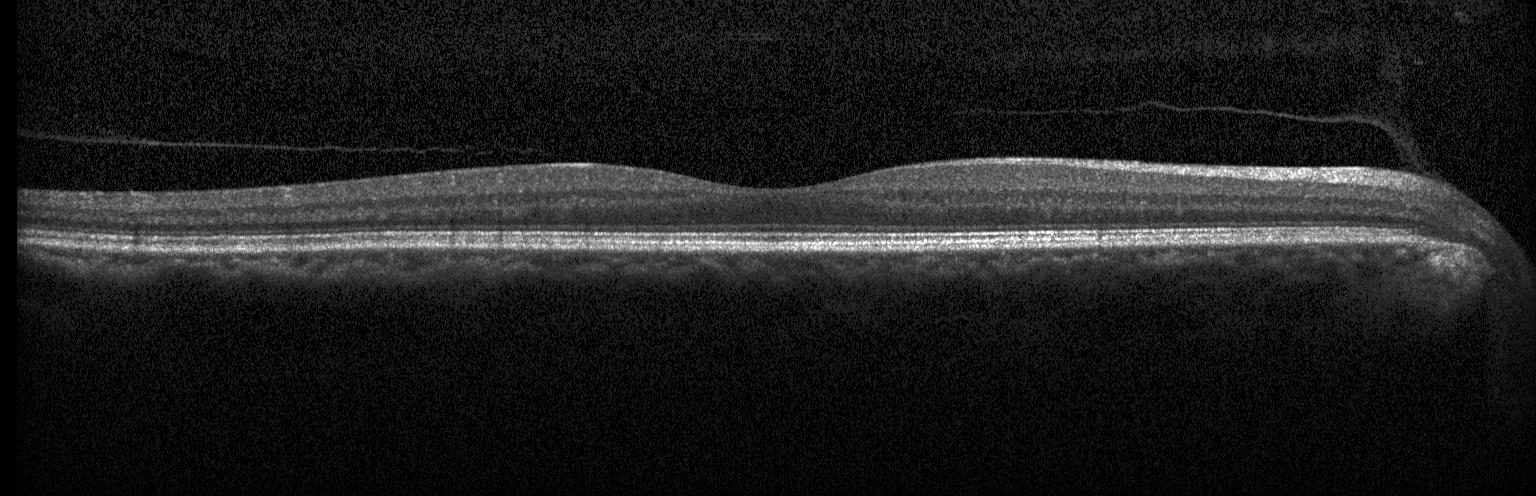

OCT finding: no choroidal neovascularization, no diabetic macular edema, and no drusen.